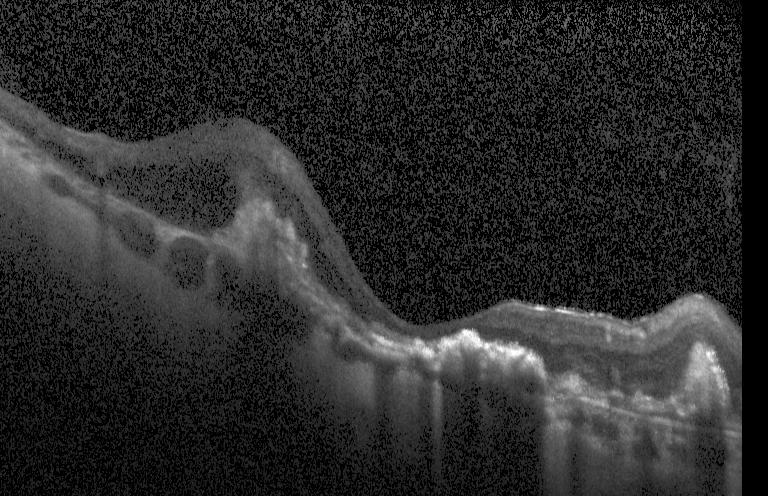 Spectral-domain optical coherence tomography, OCT B-scan, centered on the fovea — Macular OCT: a choroidal neovascular membrane.